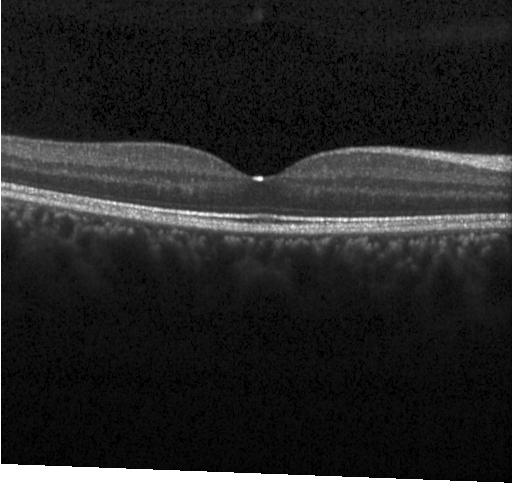
Retinal OCT cross-section showing no choroidal neovascularization, no diabetic macular edema, and no drusen.